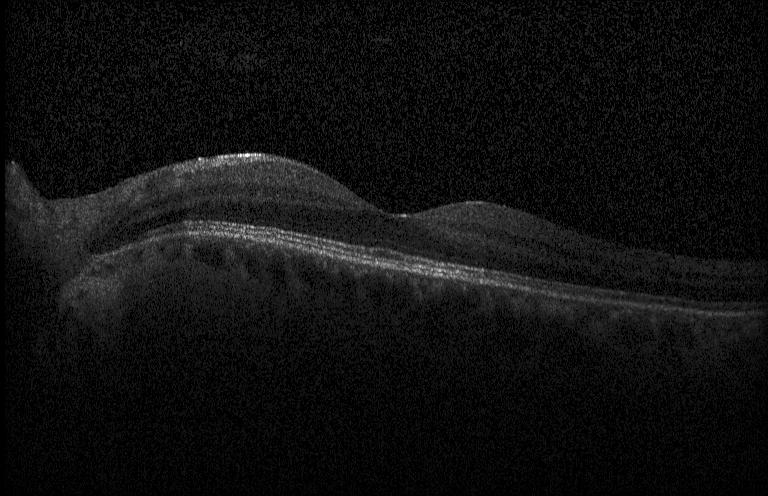 Optical coherence tomography B-scan
Impression: no choroidal neovascularization, no diabetic macular edema, and no drusen.